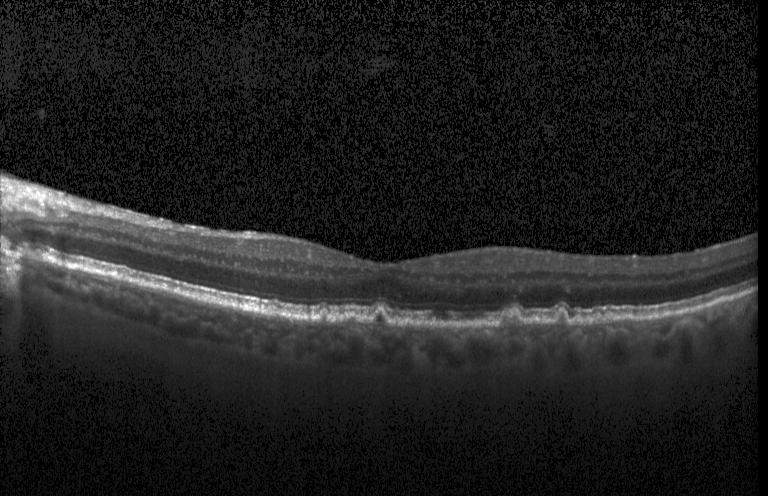
Retinal OCT B-scan · through the macula · SD-OCT
Diagnosis: drusen.